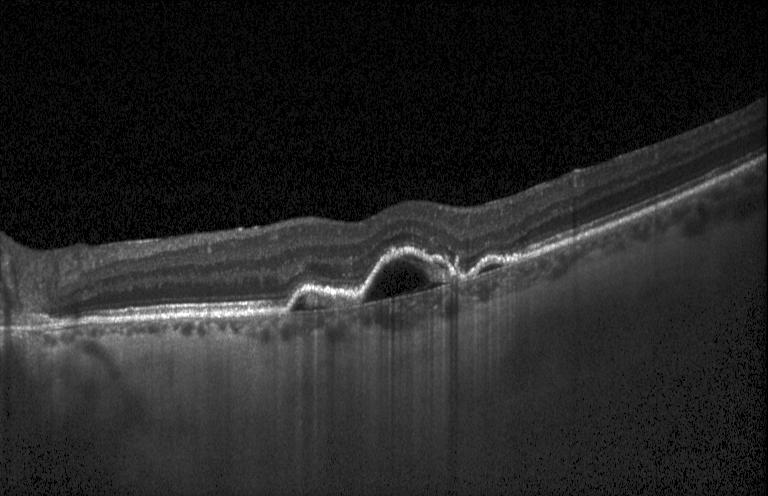
Diagnosis: a choroidal neovascular membrane.